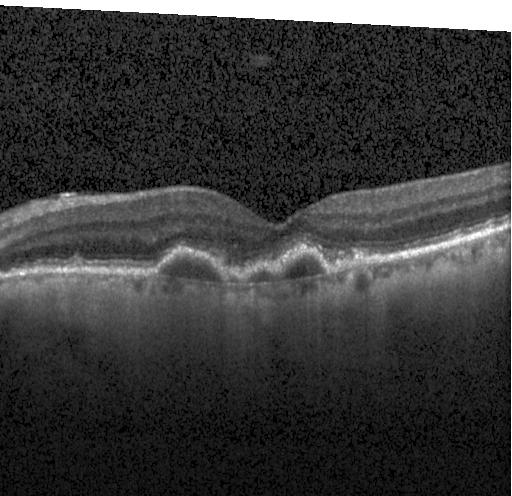
OCT line scan · instrument: Heidelberg Spectralis — Macular OCT: choroidal neovascularization.